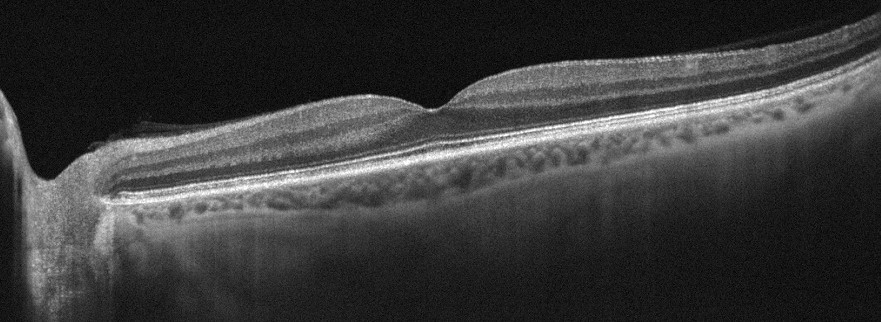 Optical coherence tomography B-scan. Fovea-centered — Assessment: absence of AMD, DME, ERM, RAO, RVO, and vitreomacular interface disease.